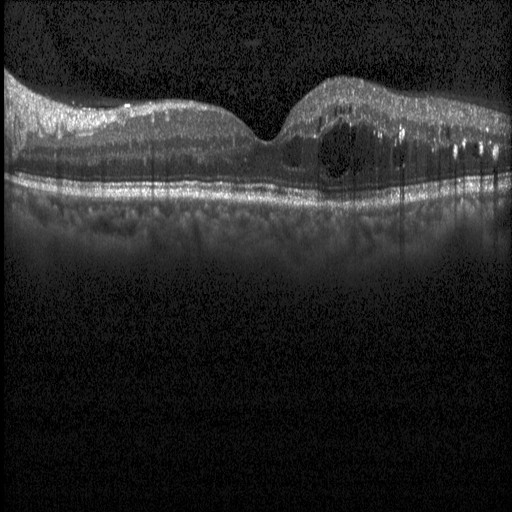

Retinal OCT B-scan — Assessment: diabetic macular edema.